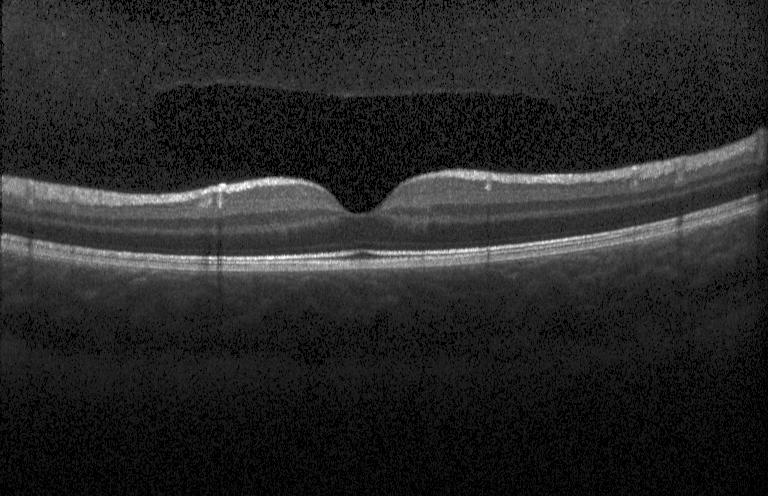

Optical coherence tomography scan. Spectral-domain optical coherence tomography. Fovea-centered. Heidelberg Spectralis
Impression: no evidence of choroidal neovascularization, diabetic macular edema, or drusen.